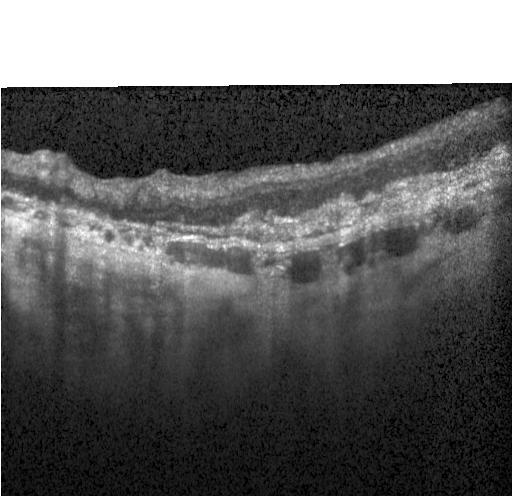 Assessment: a choroidal neovascular membrane.